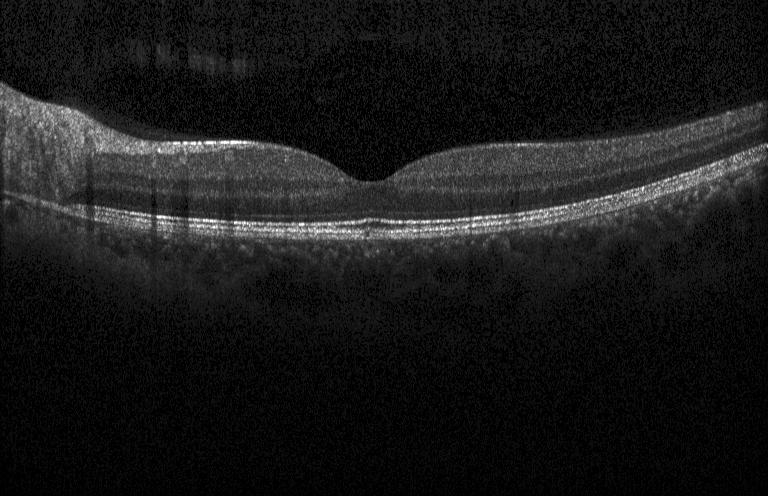

Spectral-domain optical coherence tomography, Heidelberg Spectralis, OCT B-scan, macular scan
This B-scan demonstrates no CNV, no DME, and no drusen.